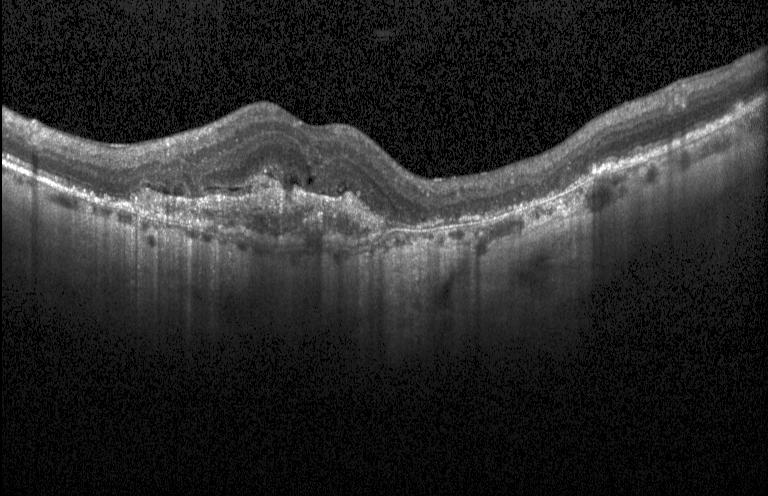 SD-OCT, through the macula, instrument: Heidelberg Spectralis, optical coherence tomography scan
Diagnosis: a choroidal neovascular membrane.